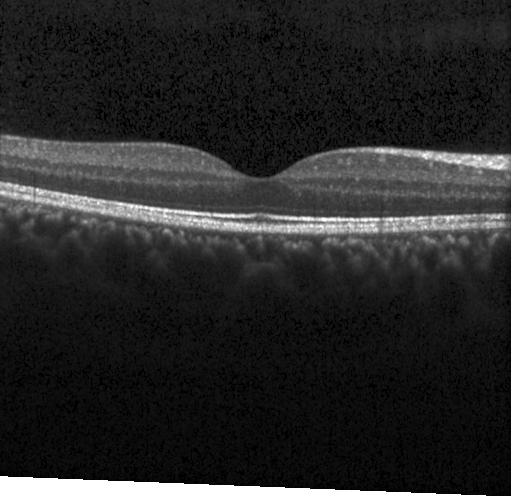
OCT scan showing no choroidal neovascularization, no diabetic macular edema, and no drusen.